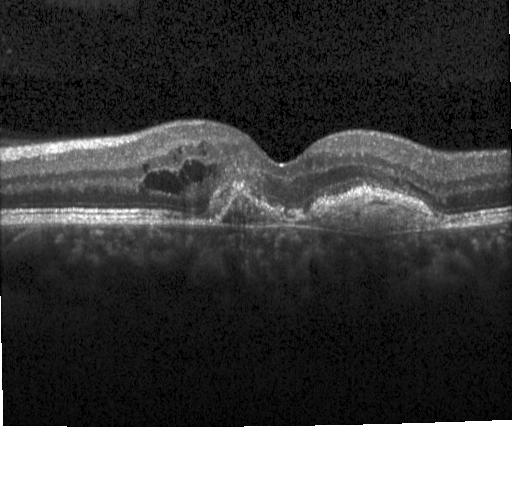
Spectral-domain OCT, centered on the fovea, retinal OCT cross-section, instrument: Heidelberg Spectralis — OCT finding: a choroidal neovascular membrane.